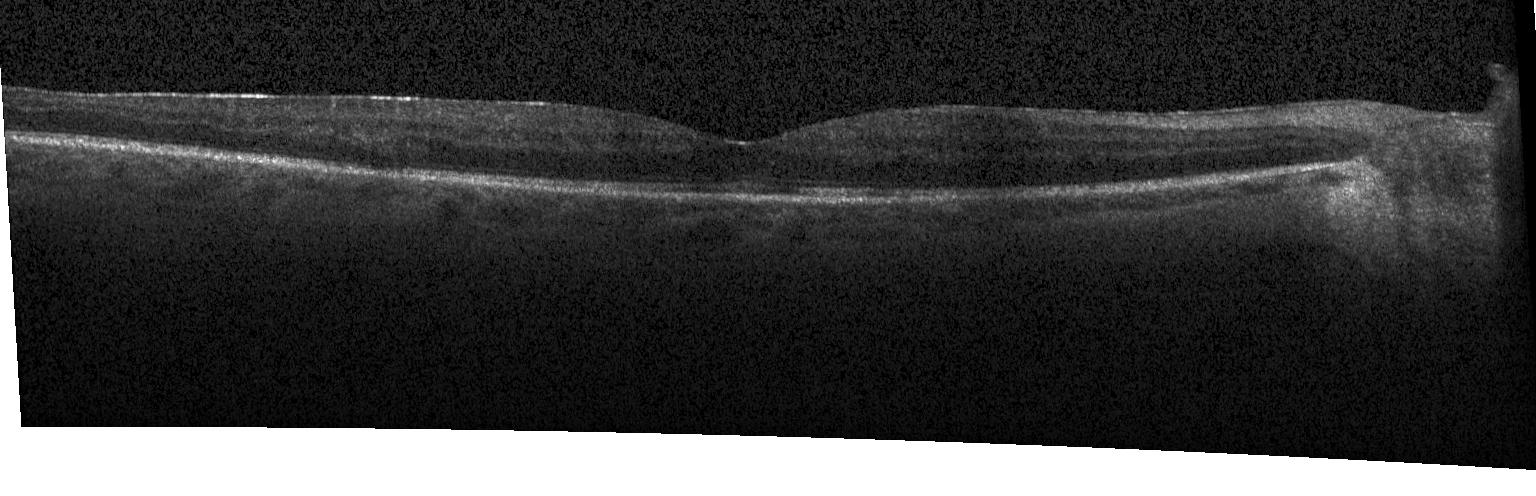 Macular scan, retinal OCT B-scan, SD-OCT.
This B-scan demonstrates no choroidal neovascularization, no diabetic macular edema, and no drusen.